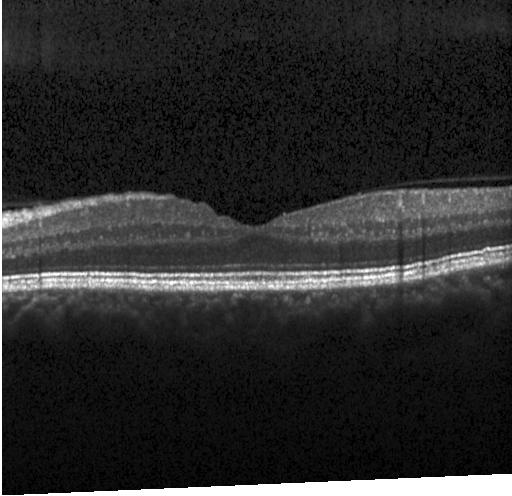
Macular scan. Optical coherence tomography scan. Spectral-domain optical coherence tomography. Heidelberg Spectralis OCT system — Impression: no evidence of choroidal neovascularization, diabetic macular edema, or drusen.